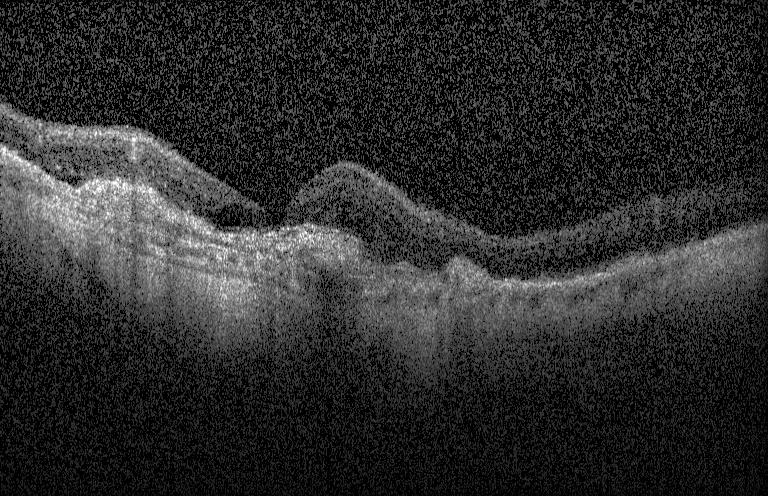

Heidelberg Spectralis. OCT B-scan. Spectral-domain OCT. Centered on the fovea
Macular OCT: a choroidal neovascular membrane.